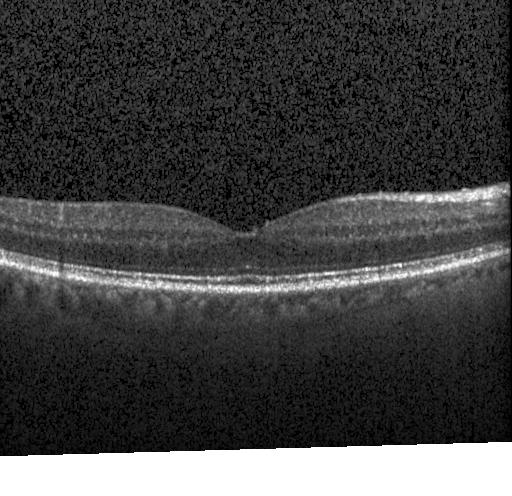

Horizontal scan through the fovea. Retinal OCT cross-section
Dx: neither choroidal neovascularization, diabetic macular edema, nor drusen.